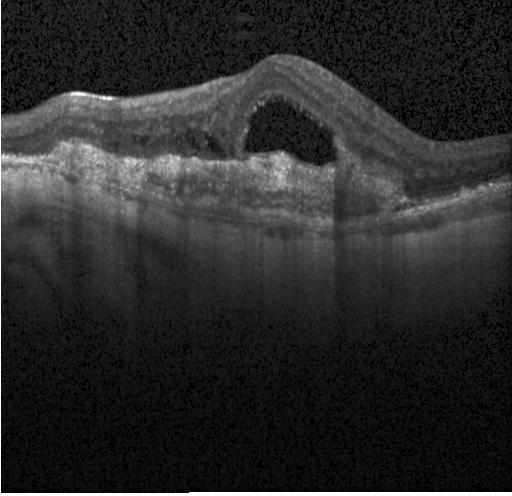
Acquired on a Heidelberg Spectralis. Fovea-centered. OCT line scan. SD-OCT
Macular OCT: choroidal neovascularization (CNV).